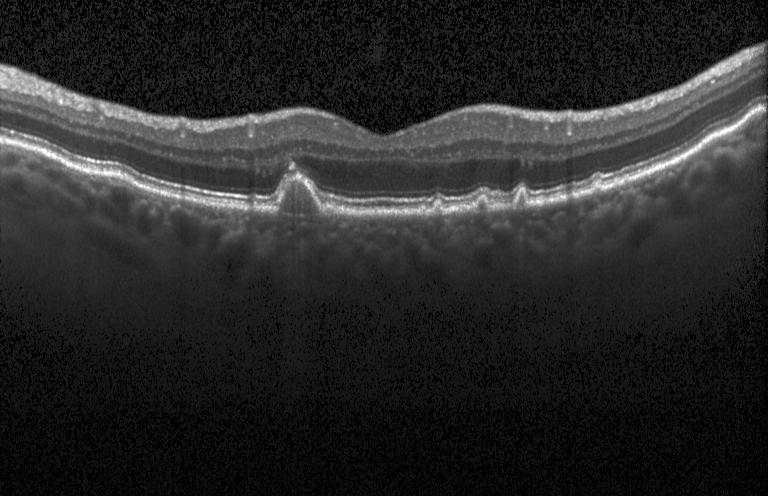
Through the macula · optical coherence tomography scan — Finding: drusen.